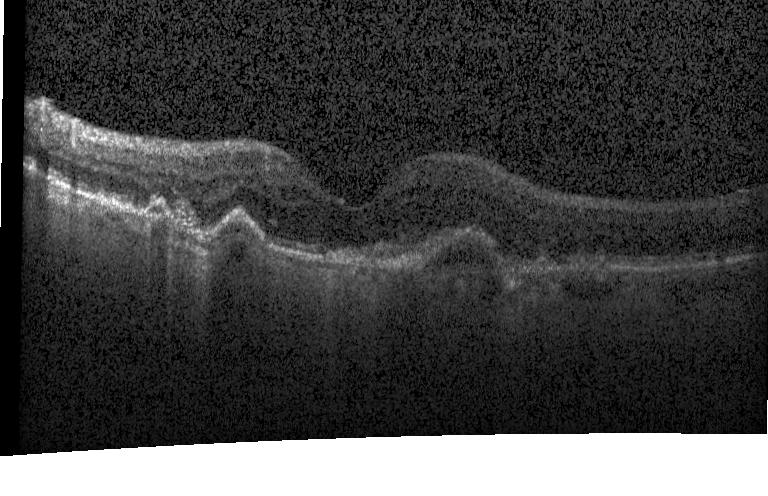
Macular OCT: CNV.